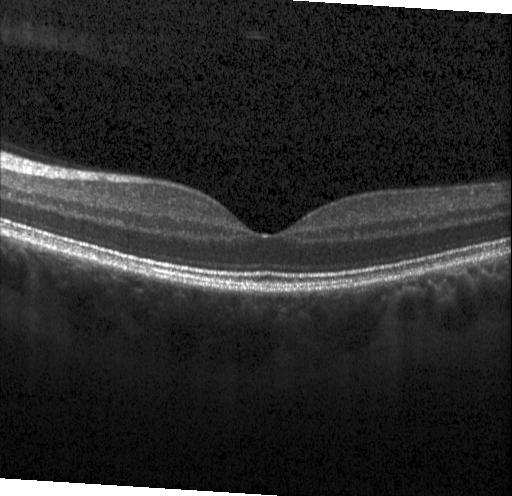 Macular OCT: no evidence of choroidal neovascularization, diabetic macular edema, or drusen.